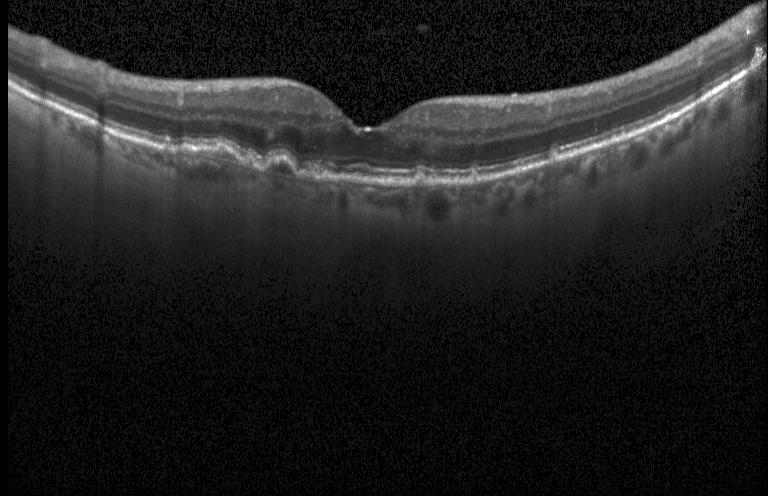 Macular OCT demonstrating multiple drusen.